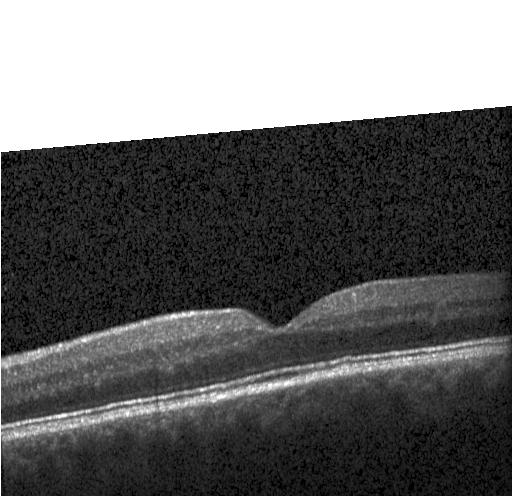
Optical coherence tomography B-scan, SD-OCT, acquired on a Heidelberg Spectralis — Diagnosis: no evidence of choroidal neovascularization, diabetic macular edema, or drusen.